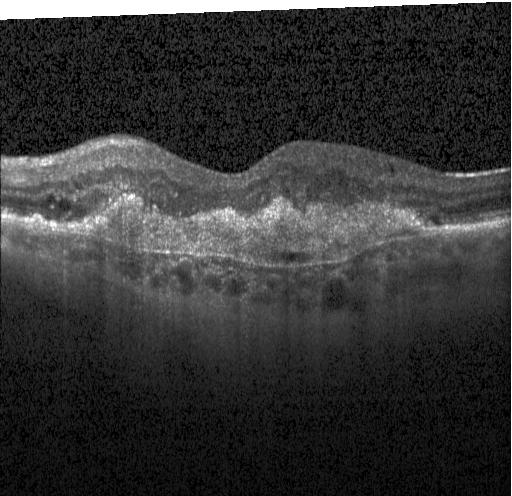
Macular scan · OCT B-scan. This B-scan demonstrates choroidal neovascularization (CNV).